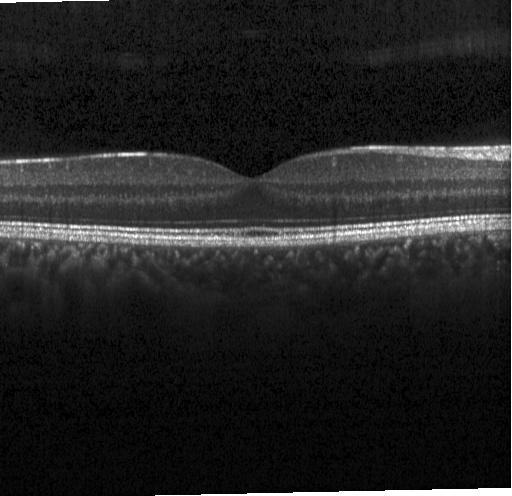

Optical coherence tomography scan — Finding: no evidence of choroidal neovascularization, diabetic macular edema, or drusen.